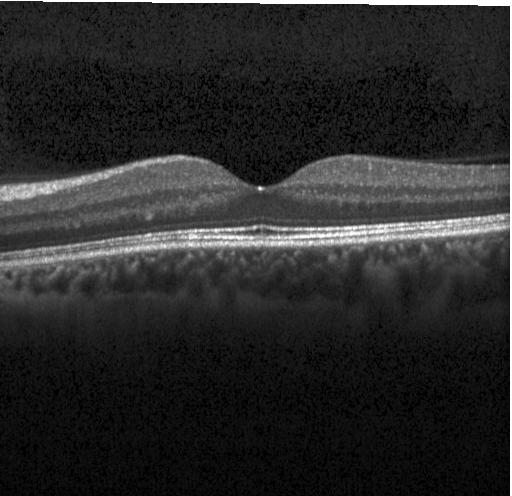
Diagnosis: no evidence of CNV, DME, or drusen.